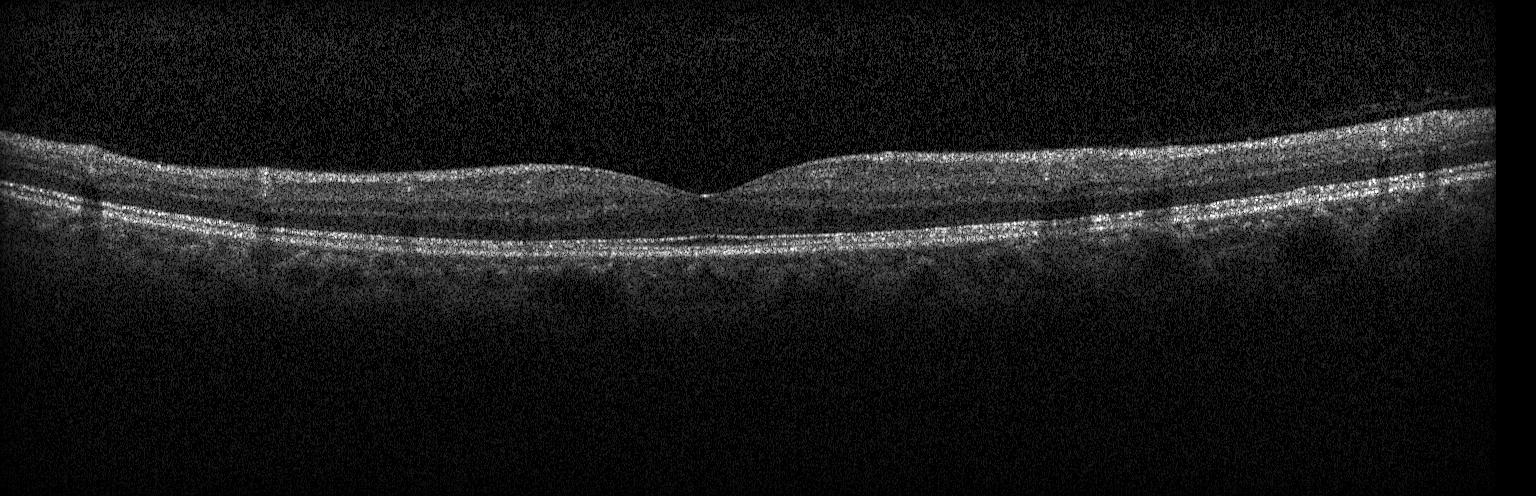
Optical coherence tomography B-scan. Spectral-domain optical coherence tomography. No choroidal neovascularization, no diabetic macular edema, and no drusen.